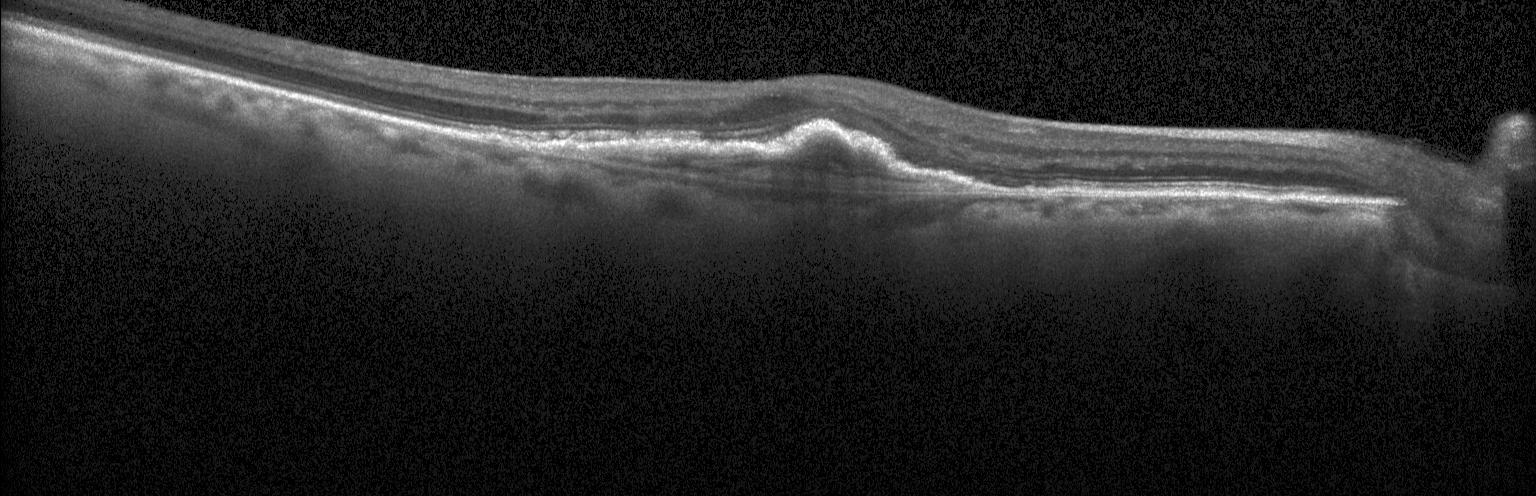

Impression: a choroidal neovascular membrane.